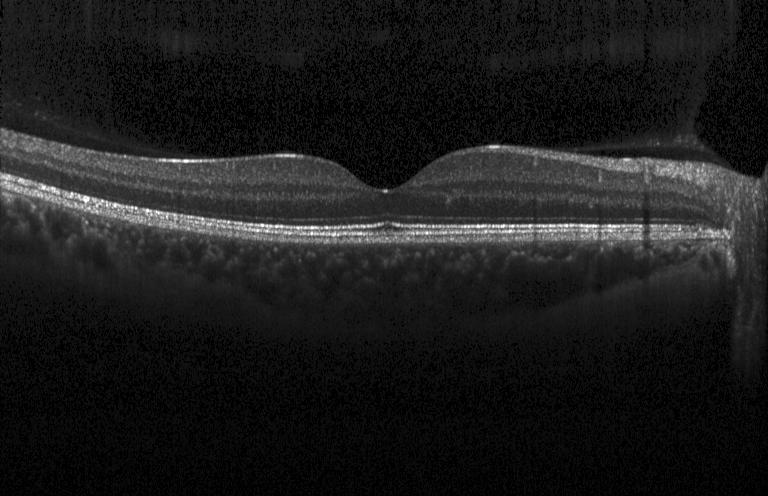
Optical coherence tomography B-scan
Diagnosis: no evidence of choroidal neovascularization, diabetic macular edema, or drusen.